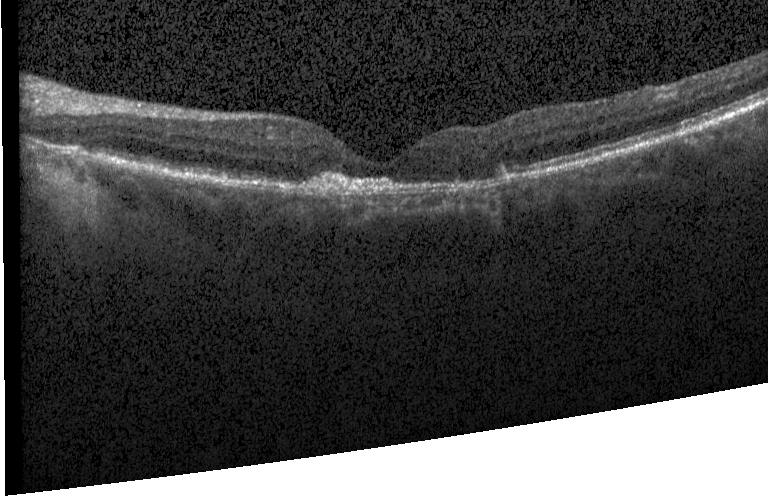
Spectral-domain optical coherence tomography. Horizontal scan through the fovea. OCT line scan. Choroidal neovascularization (CNV).